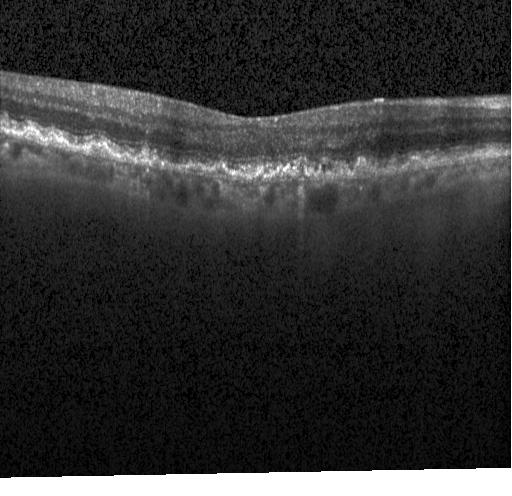
Spectral-domain OCT, centered on the fovea, acquired on a Heidelberg Spectralis, optical coherence tomography scan
This B-scan demonstrates CNV.